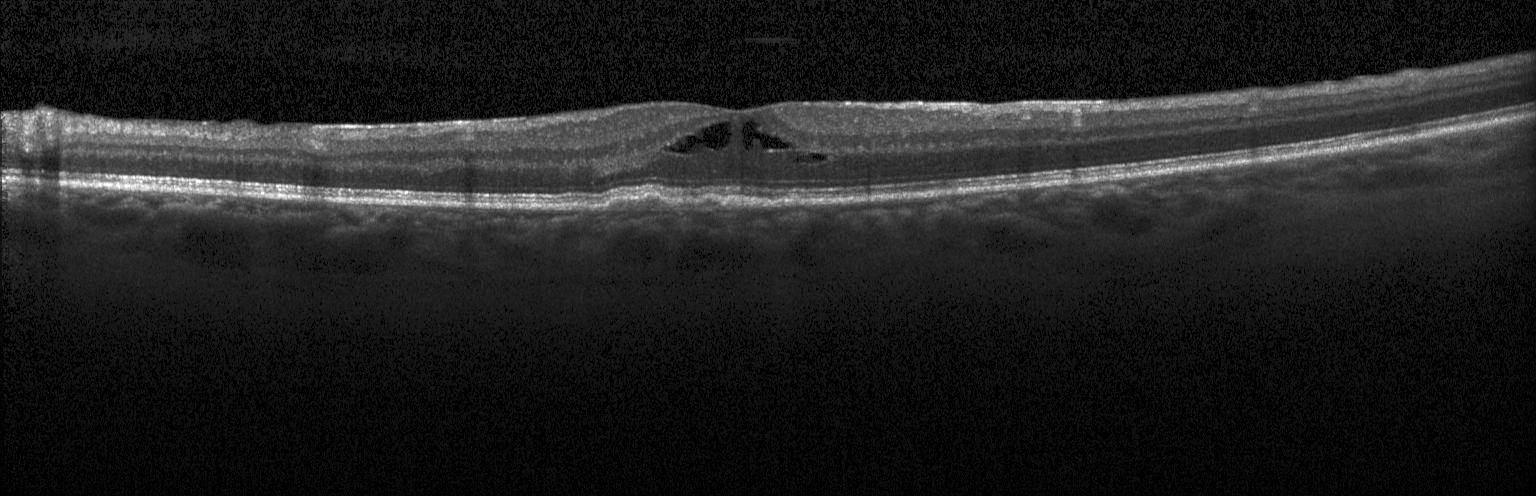 Optical coherence tomography B-scan; spectral-domain OCT; Heidelberg Spectralis; through the macula.
Diagnosis: DME.